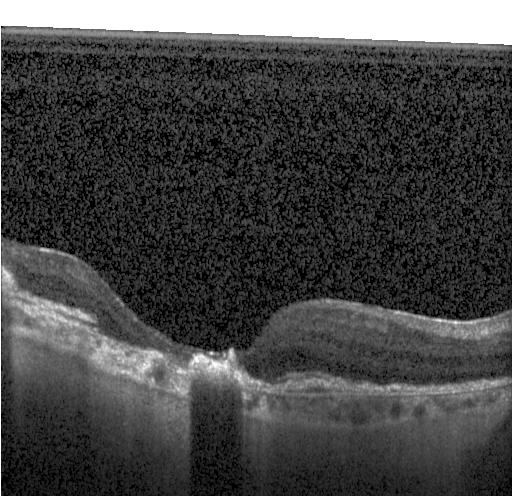
Macular scan · retinal OCT cross-section. Diagnosis: choroidal neovascularization (CNV).